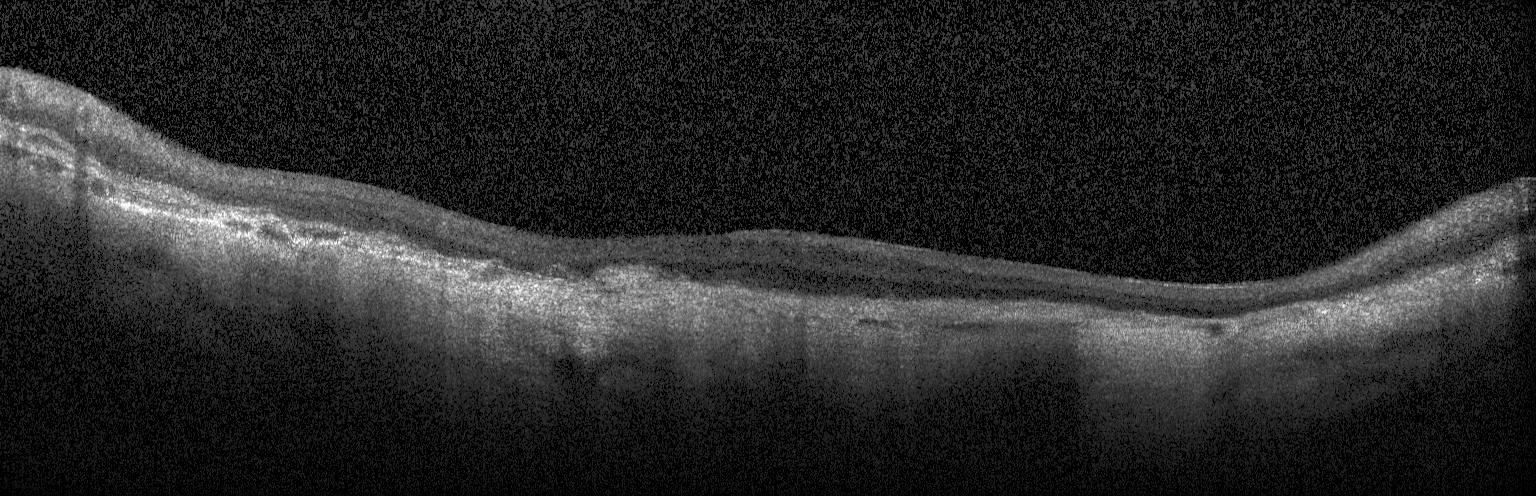

OCT line scan. Finding: a choroidal neovascular membrane.